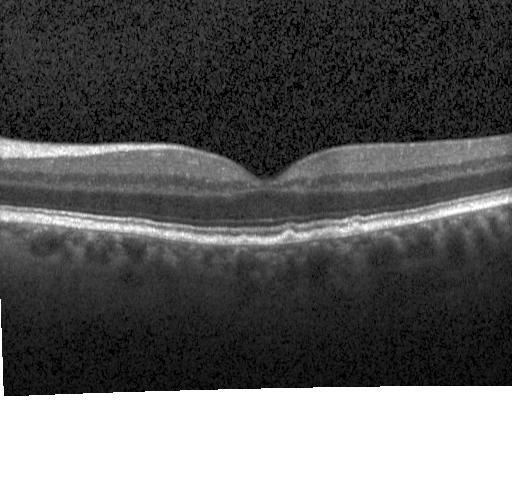
Diagnosis: drusen.